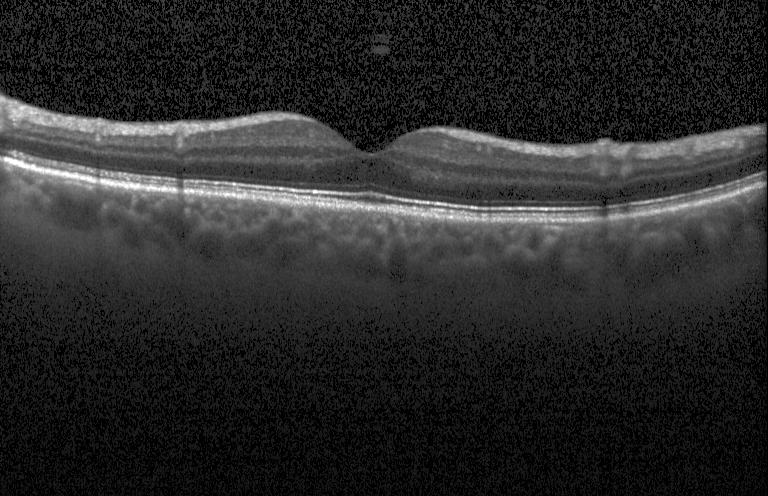
Spectral-domain OCT; retinal OCT cross-section; macular scan.
Dx: neither choroidal neovascularization, diabetic macular edema, nor drusen.